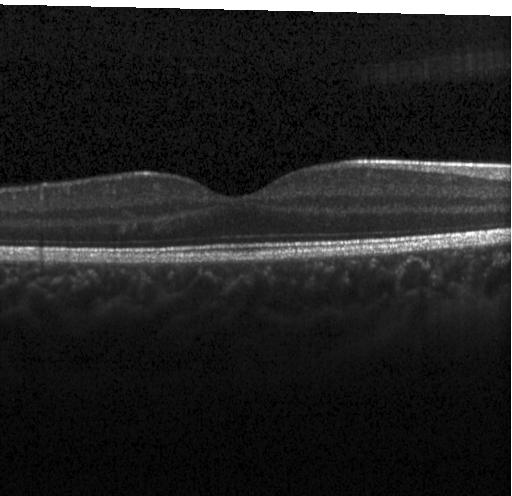 Spectral-domain OCT B-scan: no CNV, DME, or drusen.